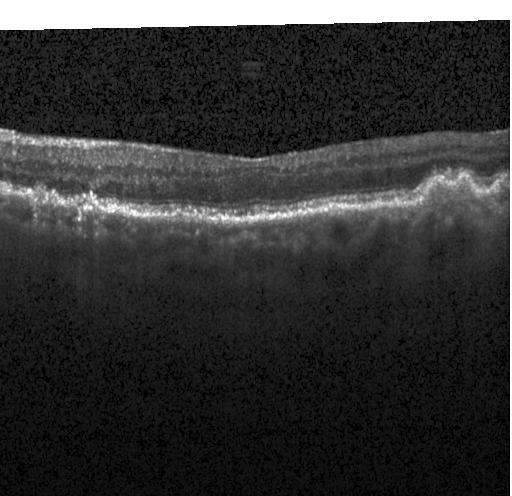 Impression: multiple drusen.